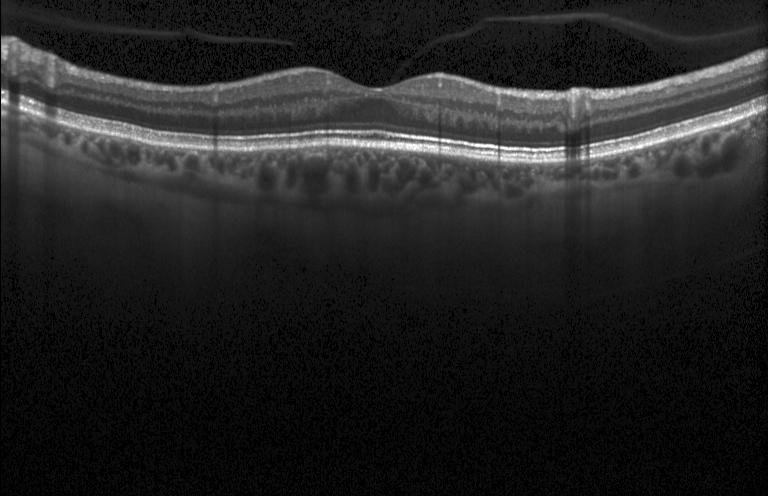

Heidelberg Spectralis OCT system · OCT B-scan · SD-OCT
Finding: no CNV, no DME, and no drusen.